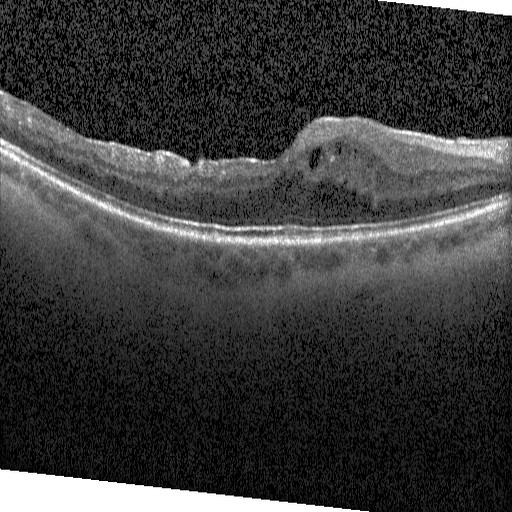 Retinal OCT cross-section, acquired on a Heidelberg Spectralis, SD-OCT, through the macula.
Assessment: DME.